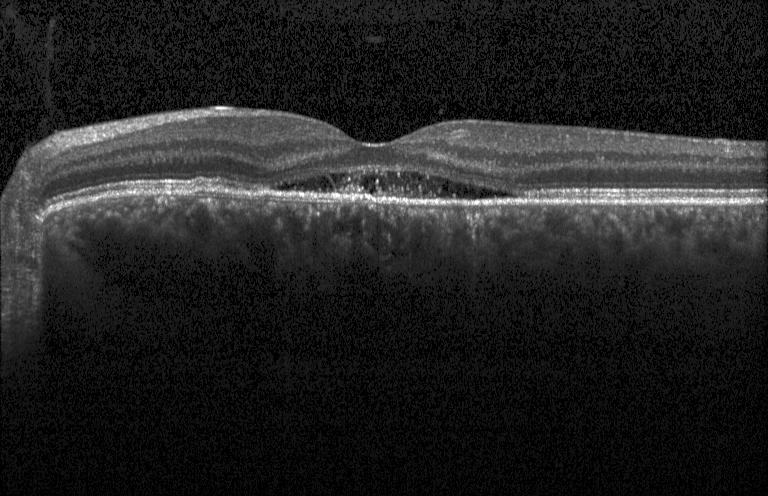
Centered on the fovea. OCT line scan. Heidelberg Spectralis OCT system. Spectral-domain optical coherence tomography — Diagnosis: a choroidal neovascular membrane.